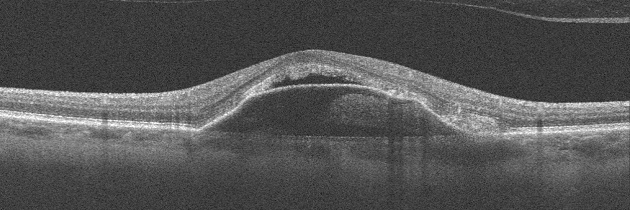
Right eye · instrument: Optovue Avanti RTVue XR · OCT line scan. Finding: age-related macular degeneration (AMD).